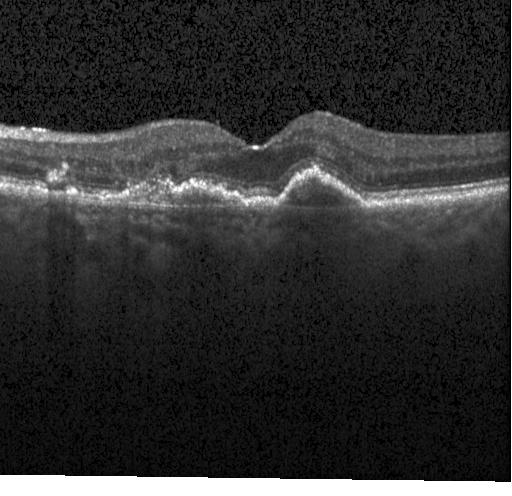

Retinal OCT cross-section
Dx: choroidal neovascularization (CNV).